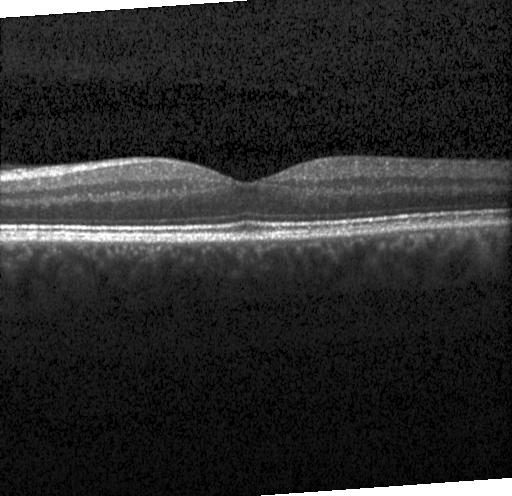

Retinal OCT cross-section. Centered on the fovea
Impression: no CNV, no DME, and no drusen.